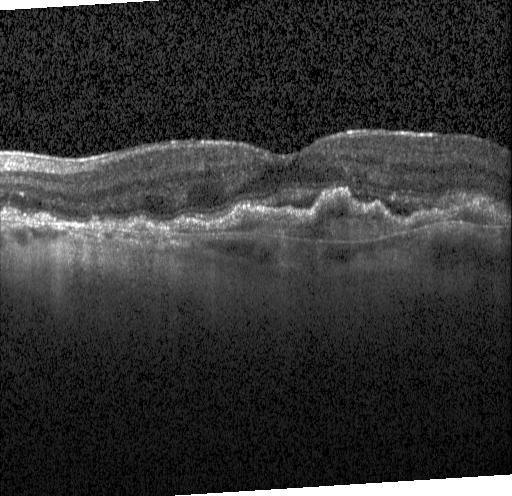
Diagnosis: CNV.